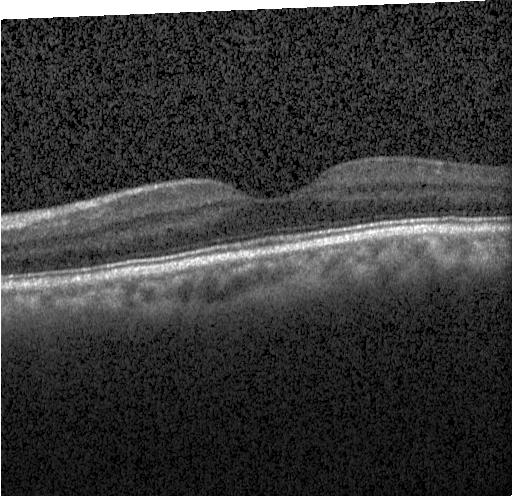

Spectral-domain OCT B-scan: no choroidal neovascularization, no diabetic macular edema, and no drusen.